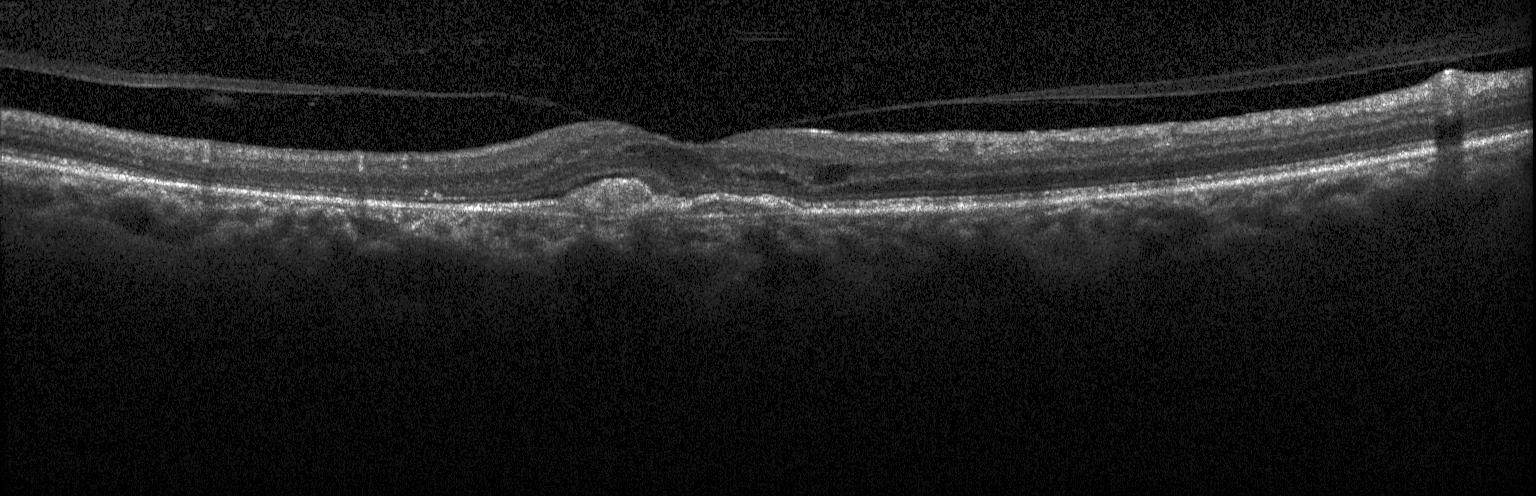
Optical coherence tomography B-scan. Acquired on a Heidelberg Spectralis. SD-OCT. Macular OCT: choroidal neovascularization.